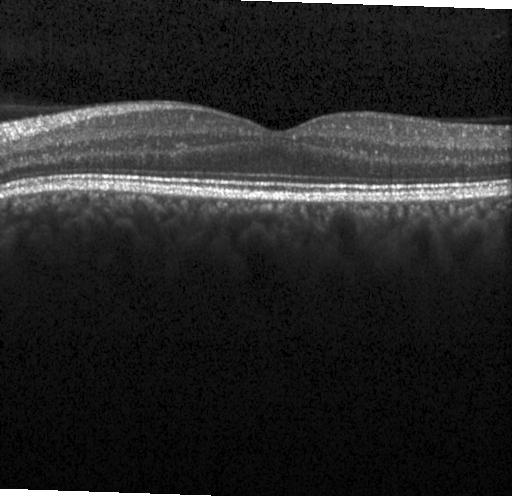 SD-OCT · retinal OCT B-scan. Diagnosis: neither CNV, DME, nor drusen.